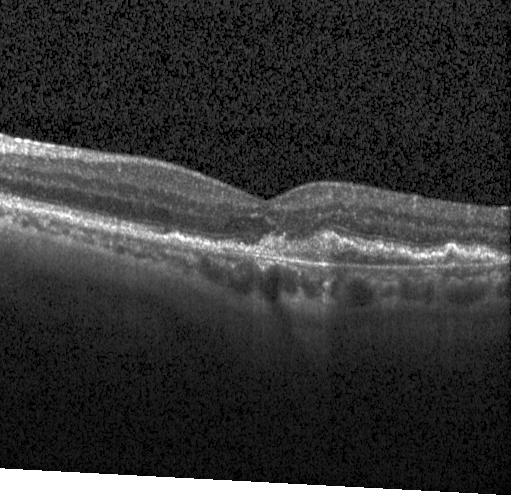
Assessment: a choroidal neovascular membrane.